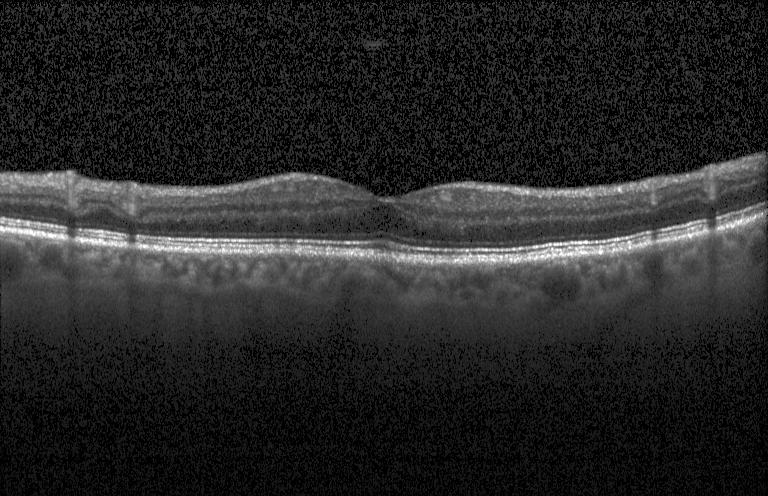 Dx: neither choroidal neovascularization, diabetic macular edema, nor drusen.